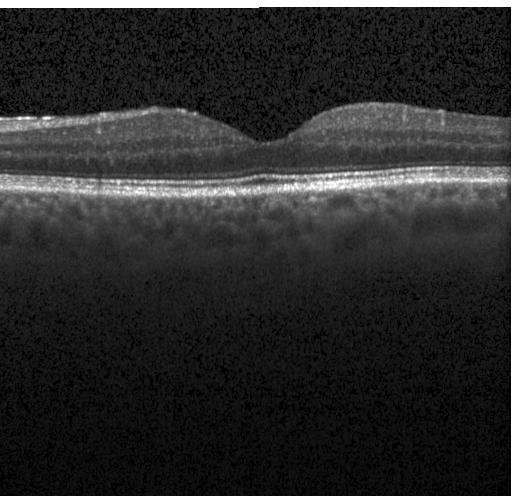 Instrument: Heidelberg Spectralis. Retinal OCT B-scan. This B-scan demonstrates no evidence of choroidal neovascularization, diabetic macular edema, or drusen.